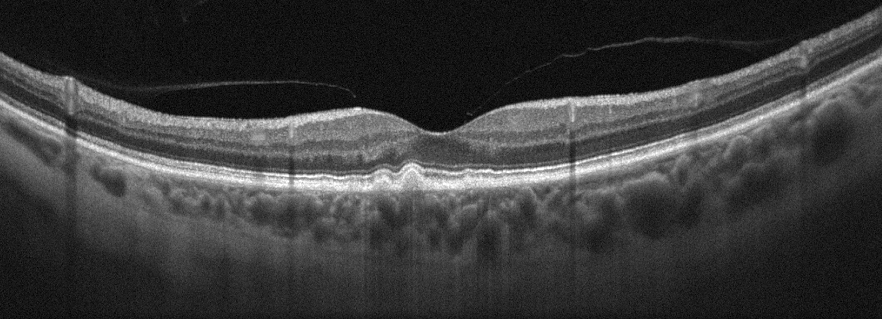 Through the macula, OCT line scan
The scan shows age-related macular degeneration (AMD).